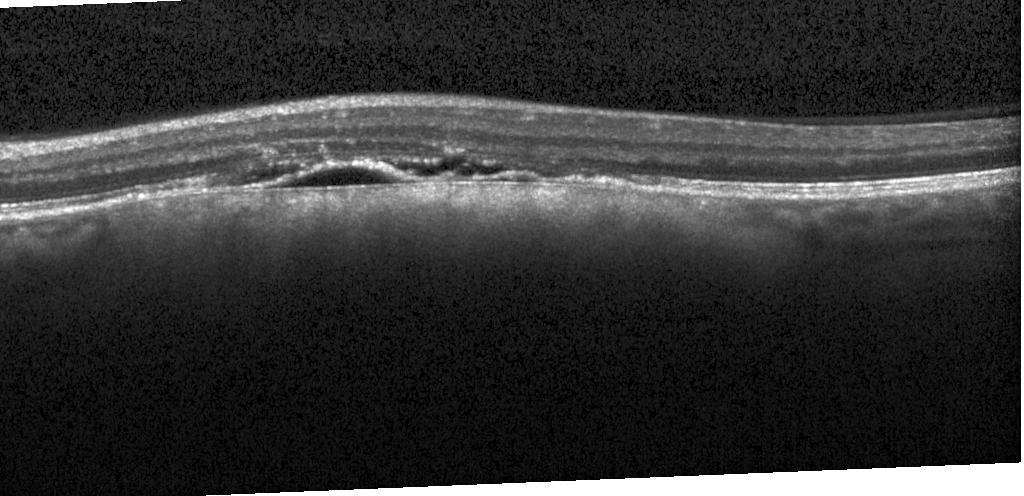 Retinal OCT cross-section. Spectral-domain OCT. Acquired on a Heidelberg Spectralis. Fovea-centered.
Finding: choroidal neovascularization (CNV).